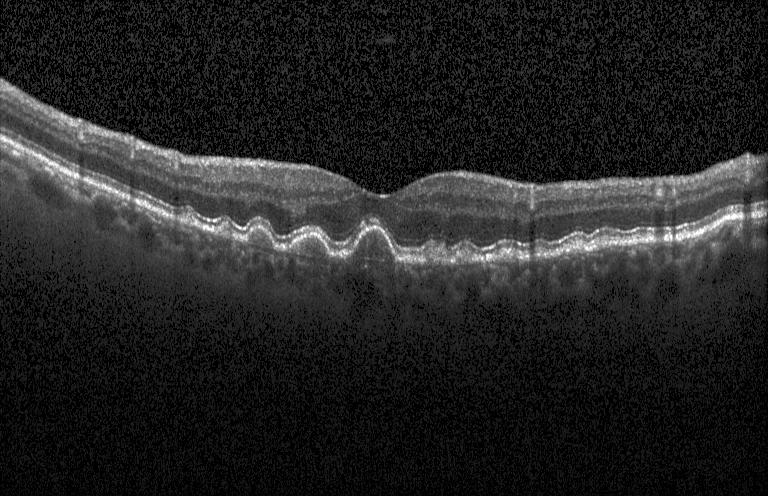

Heidelberg Spectralis. Centered on the fovea. OCT line scan. Spectral-domain OCT. Finding: sub-RPE drusenoid deposits.